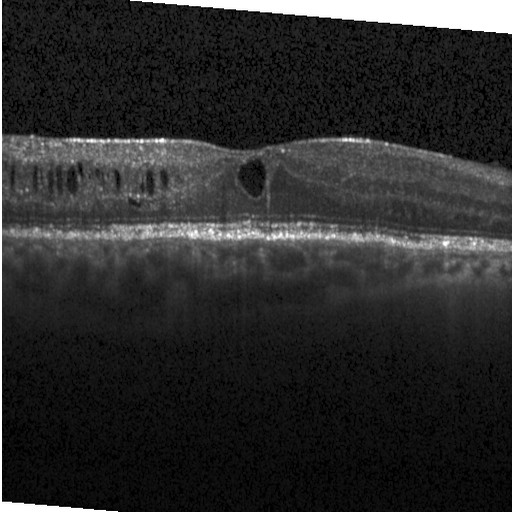

Macular scan; spectral-domain optical coherence tomography; OCT line scan.
Finding: diabetic macular edema (DME).